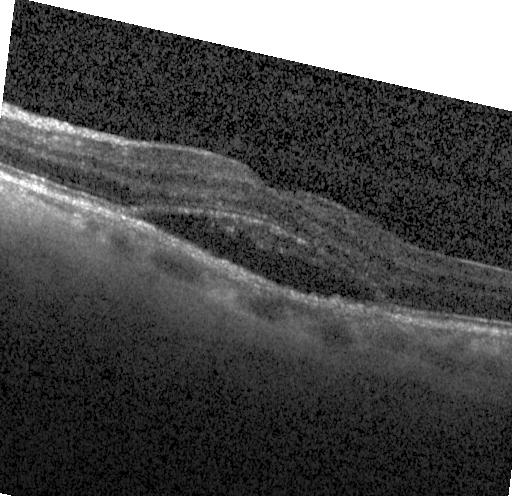

Retinal OCT cross-section — Assessment: choroidal neovascularization (CNV).